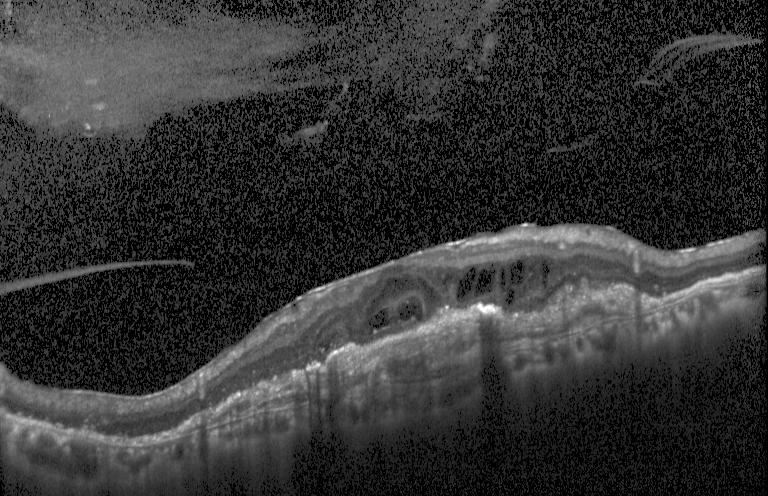
Through the macula · SD-OCT · OCT line scan
Diagnosis: a choroidal neovascular membrane.